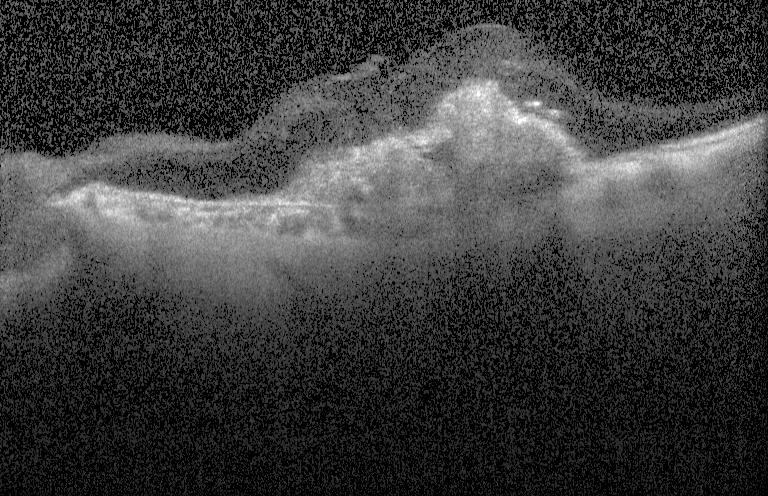

OCT B-scan showing CNV.